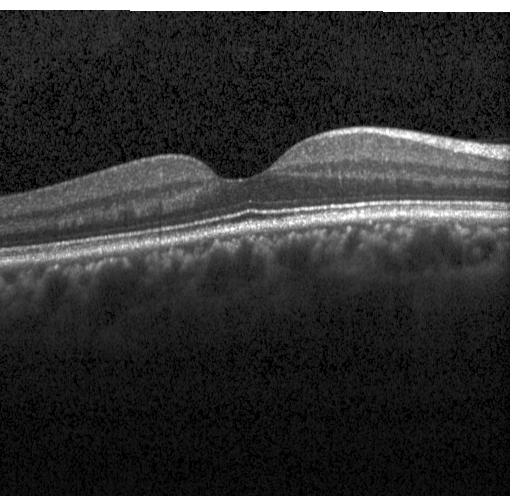
Retinal OCT B-scan · spectral-domain OCT — This B-scan demonstrates no evidence of choroidal neovascularization, diabetic macular edema, or drusen.